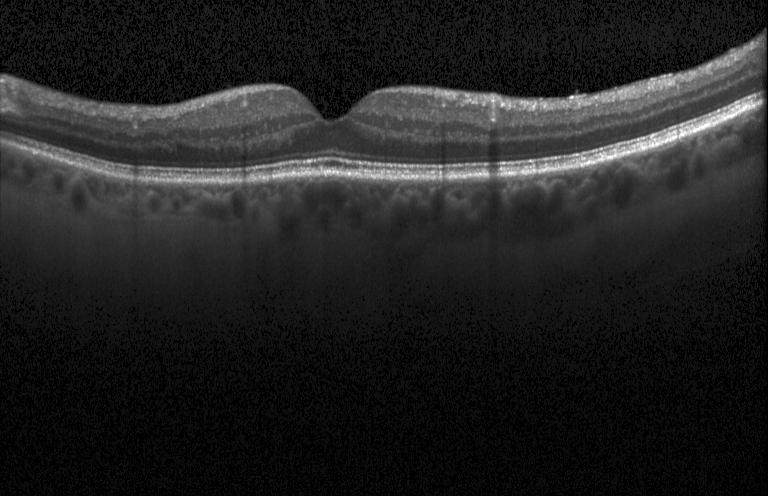

Acquired on a Heidelberg Spectralis · retinal OCT cross-section — The scan shows no choroidal neovascularization, no diabetic macular edema, and no drusen.